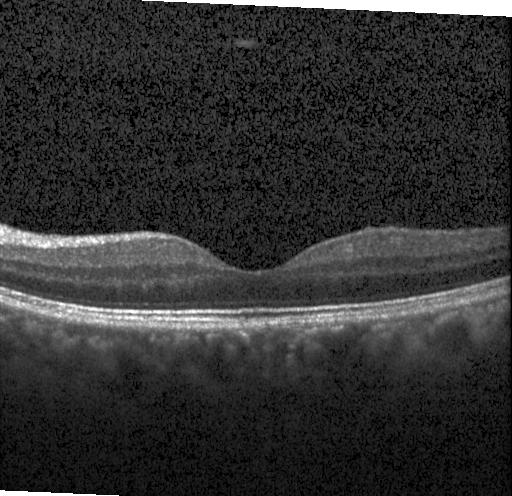 Finding: neither CNV, DME, nor drusen.